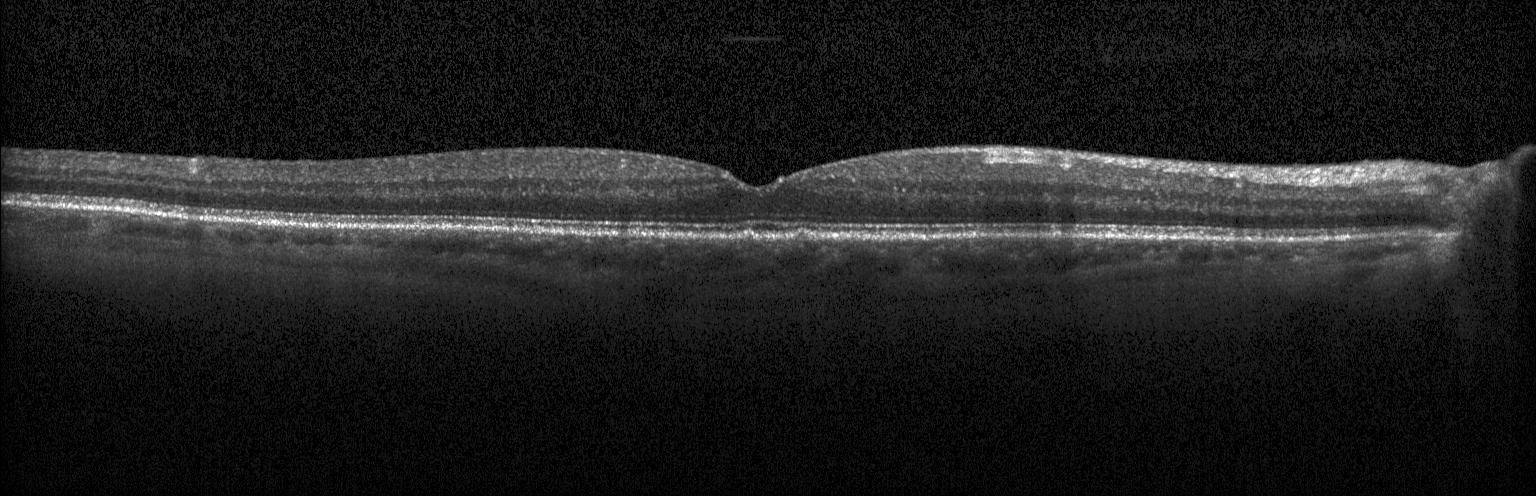 Instrument: Heidelberg Spectralis. Macular scan. OCT B-scan. Spectral-domain optical coherence tomography.
Assessment: sub-RPE drusenoid deposits.